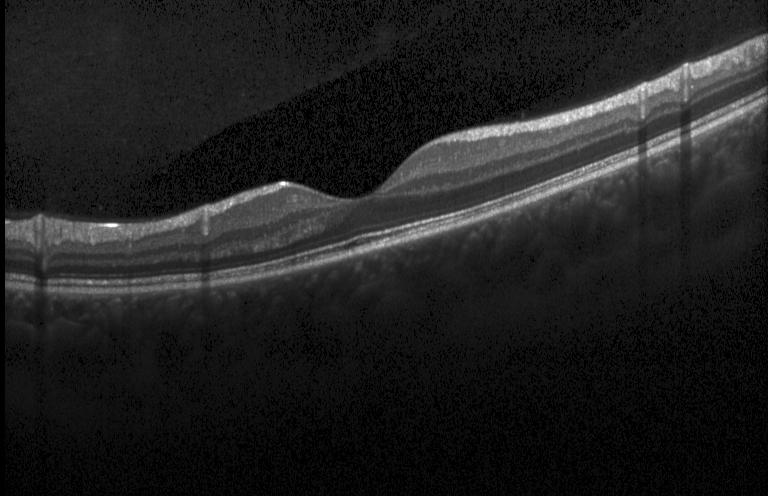
Spectral-domain optical coherence tomography. Macular scan. OCT B-scan. Heidelberg Spectralis OCT system — Diagnosis: no choroidal neovascularization, no diabetic macular edema, and no drusen.